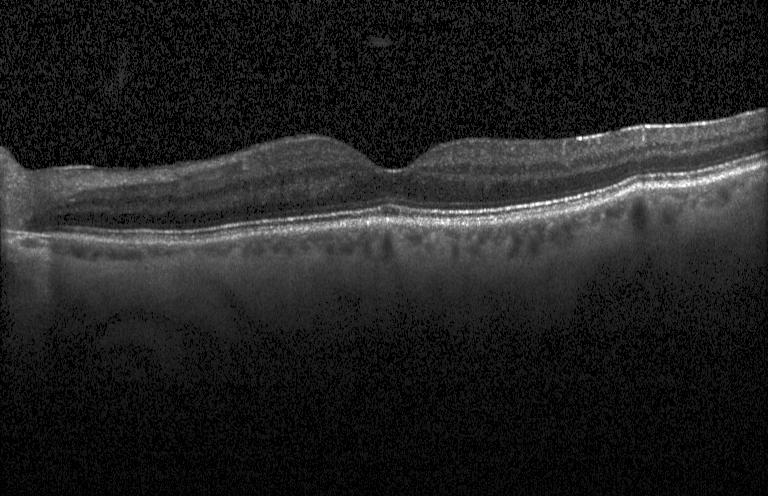
Horizontal scan through the fovea, retinal OCT cross-section, Heidelberg Spectralis OCT system.
Finding: no choroidal neovascularization, no diabetic macular edema, and no drusen.